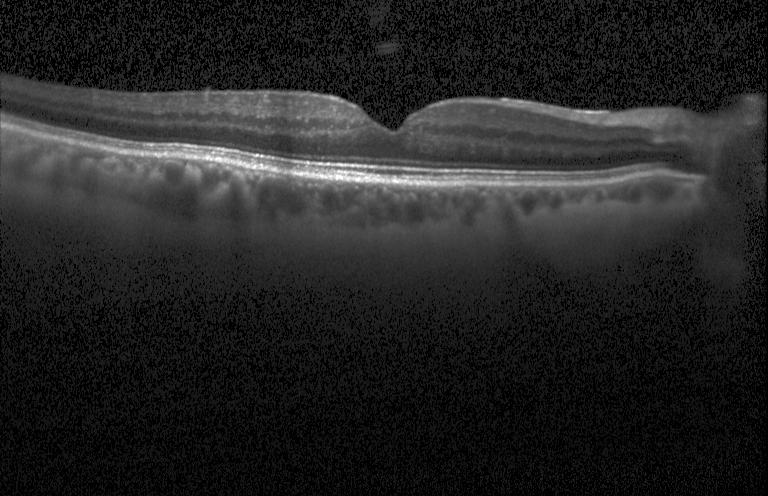
Retinal OCT B-scan — Finding: no evidence of choroidal neovascularization, diabetic macular edema, or drusen.